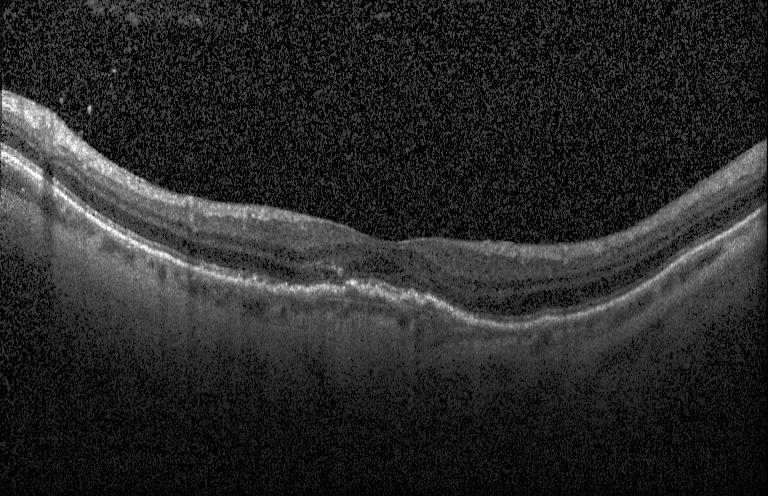 Retinal OCT cross-section showing choroidal neovascularization.